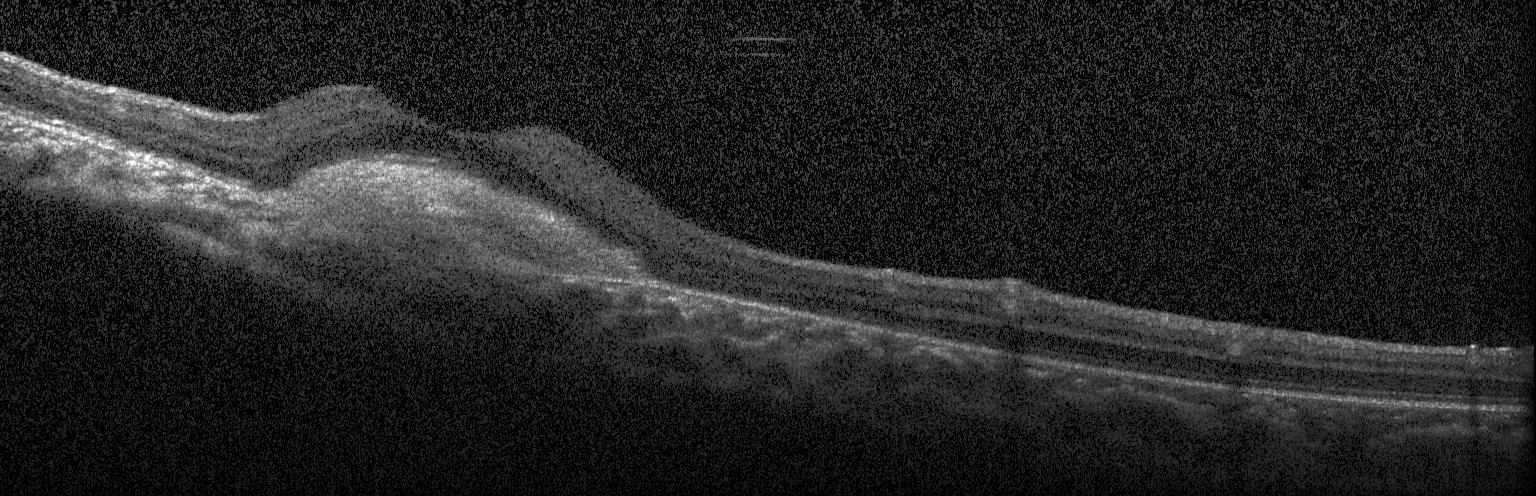

Retinal OCT cross-section showing a choroidal neovascular membrane.